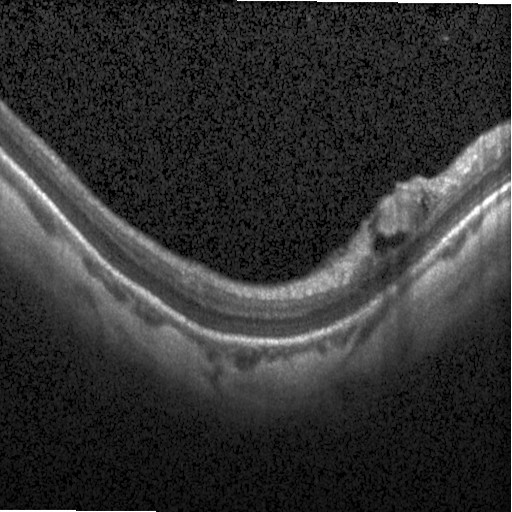

DME.